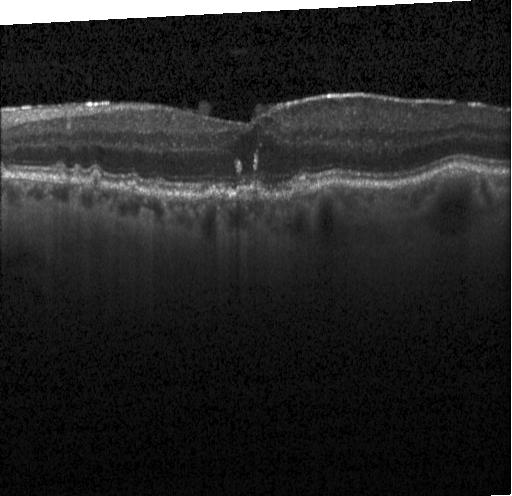 This B-scan demonstrates multiple drusen.